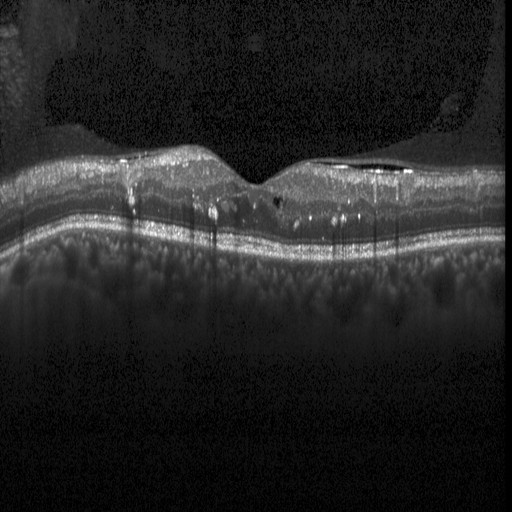

Macular scan · spectral-domain OCT · retinal OCT cross-section
Dx: diabetic macular edema (DME).